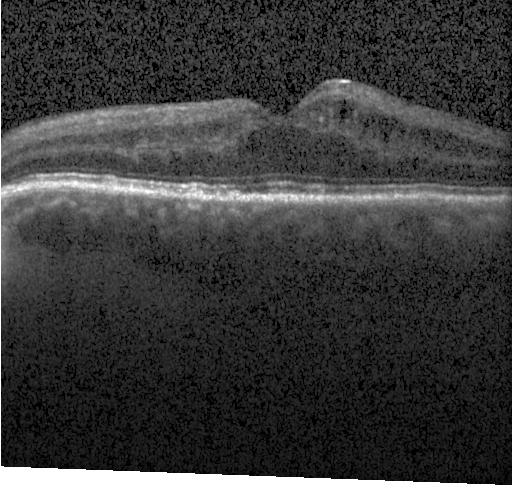 Retinal OCT B-scan. The scan shows DME.